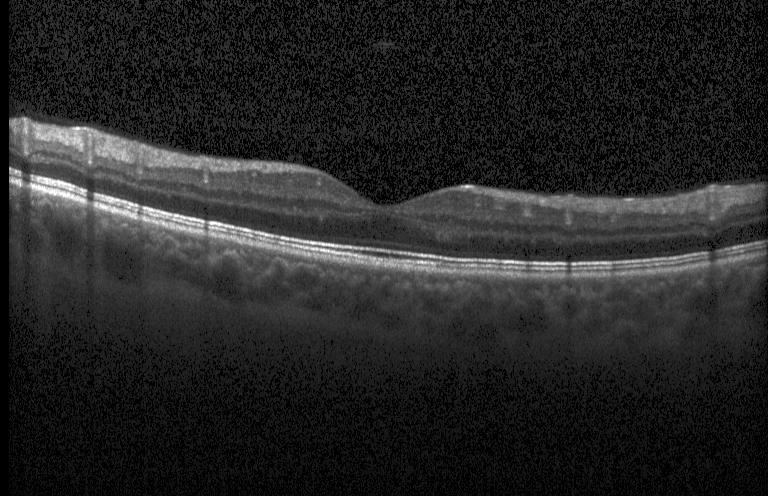

Centered on the fovea, spectral-domain optical coherence tomography, OCT line scan — The scan shows no CNV, DME, or drusen.